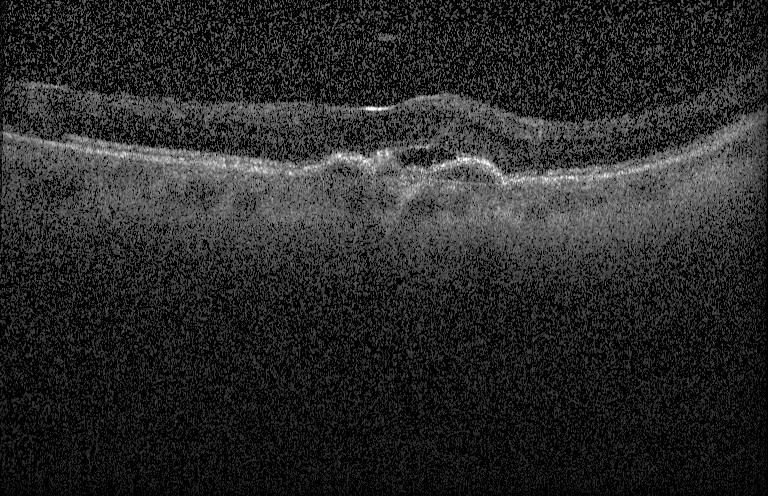

Dx: choroidal neovascularization (CNV).